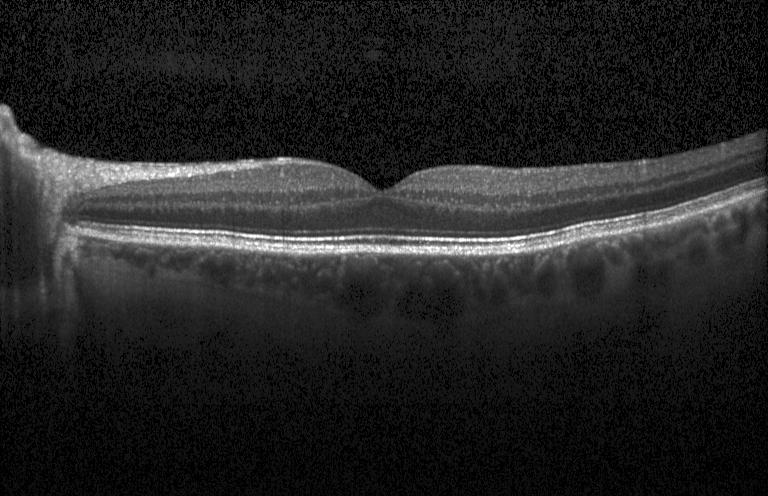 Macular OCT: no choroidal neovascularization, diabetic macular edema, or drusen.